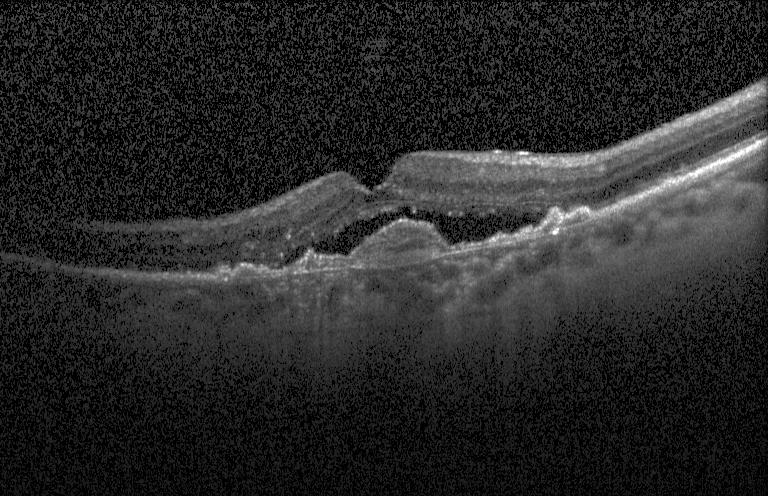
SD-OCT. Optical coherence tomography scan. Horizontal scan through the fovea
A choroidal neovascular membrane.